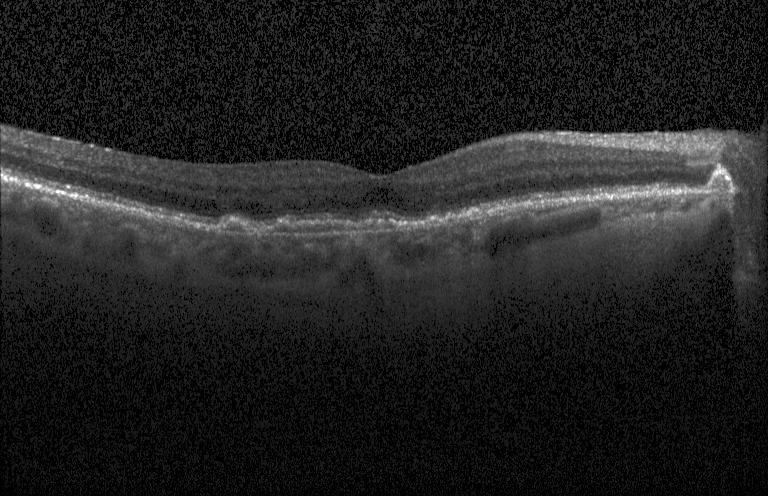

OCT B-scan showing CNV.